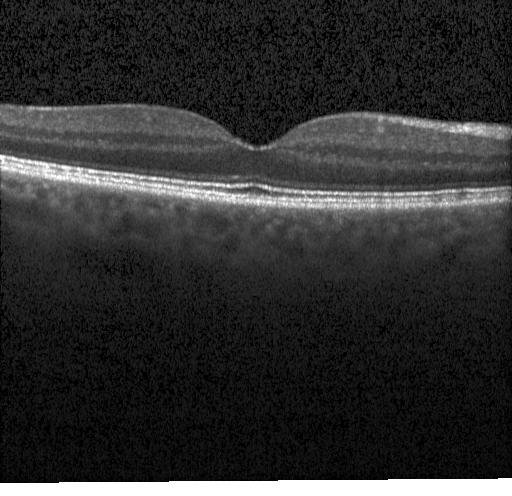 Heidelberg Spectralis, retinal OCT B-scan
Dx: no choroidal neovascularization, no diabetic macular edema, and no drusen.